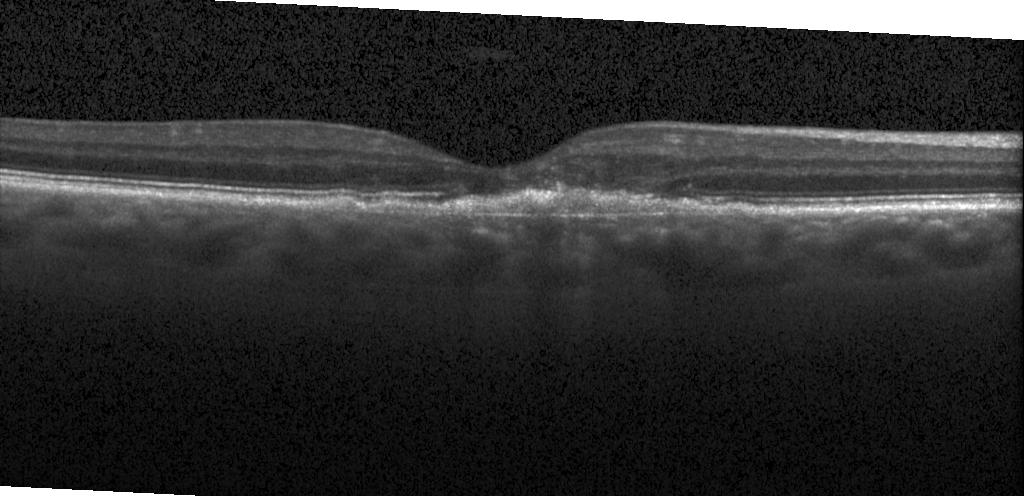
Centered on the fovea; optical coherence tomography B-scan; spectral-domain OCT — Finding: a choroidal neovascular membrane.